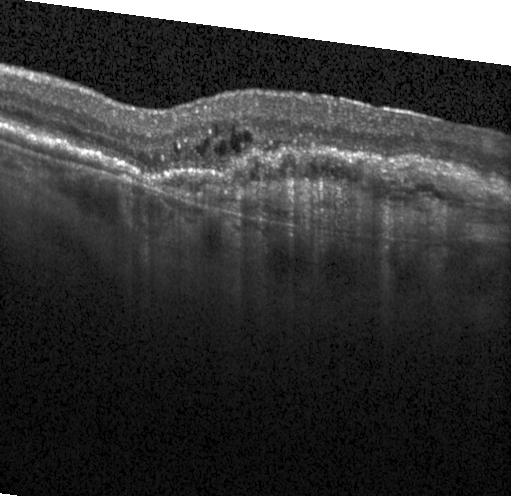 Macular OCT demonstrating choroidal neovascularization (CNV).